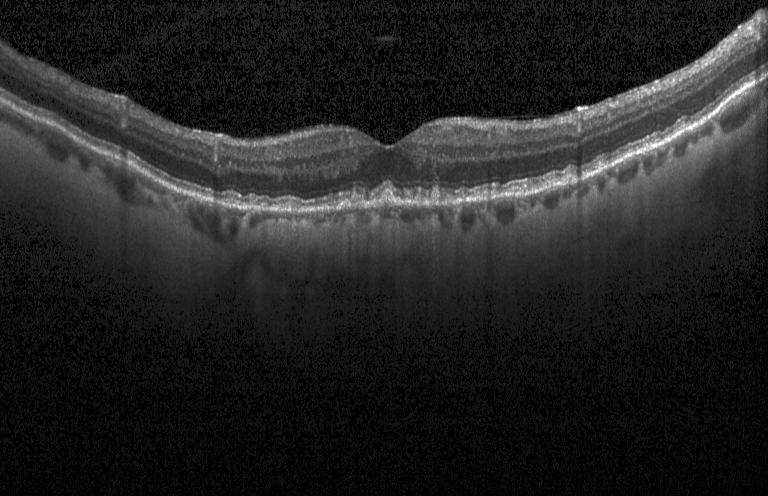 Retinal OCT cross-section; spectral-domain optical coherence tomography.
This B-scan demonstrates drusen.